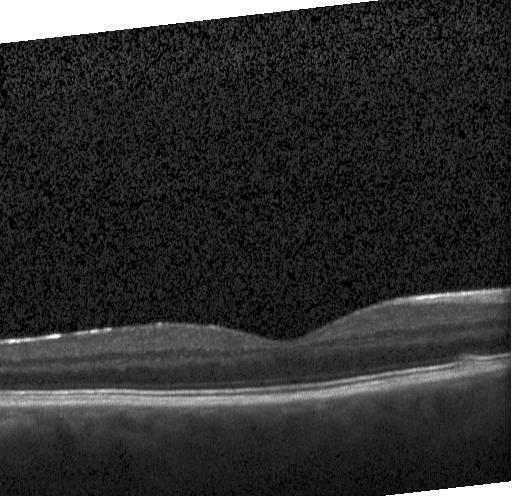

Diagnosis: multiple drusen.